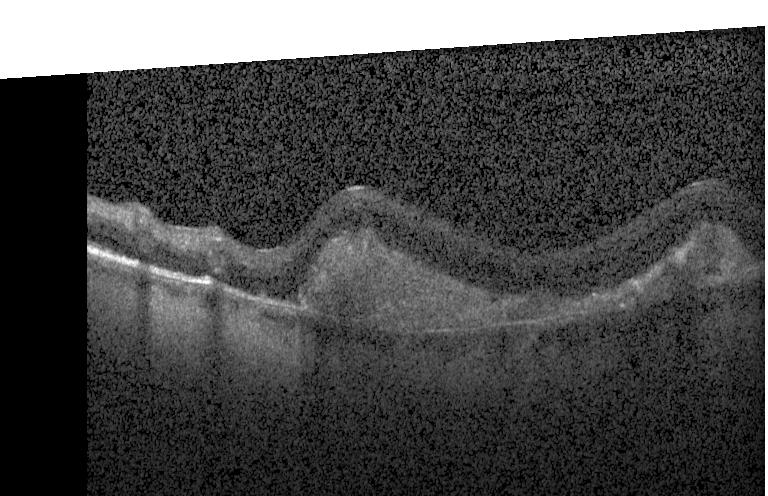
Diagnosis: a choroidal neovascular membrane.